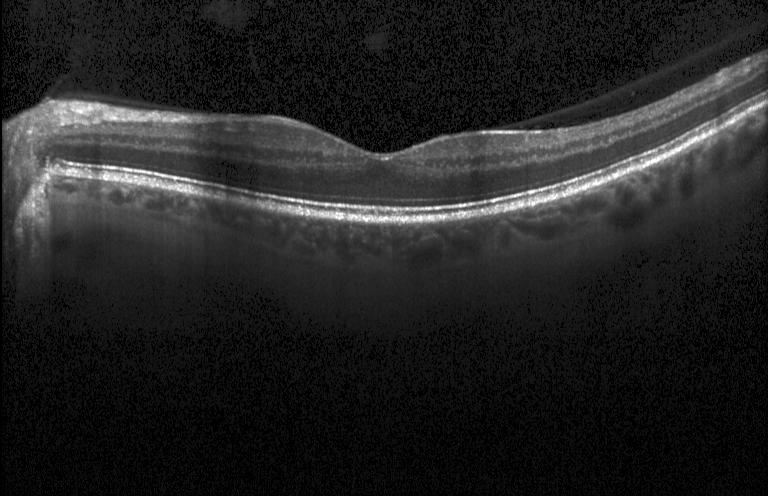 Spectral-domain optical coherence tomography. Macular scan. OCT B-scan. Heidelberg Spectralis OCT system — Dx: neither CNV, DME, nor drusen.